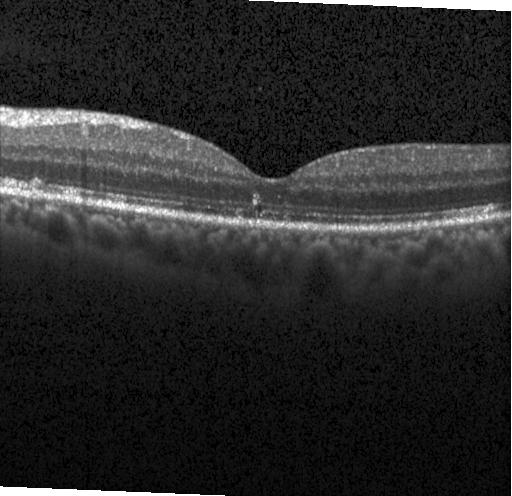

OCT B-scan showing neither CNV, DME, nor drusen.